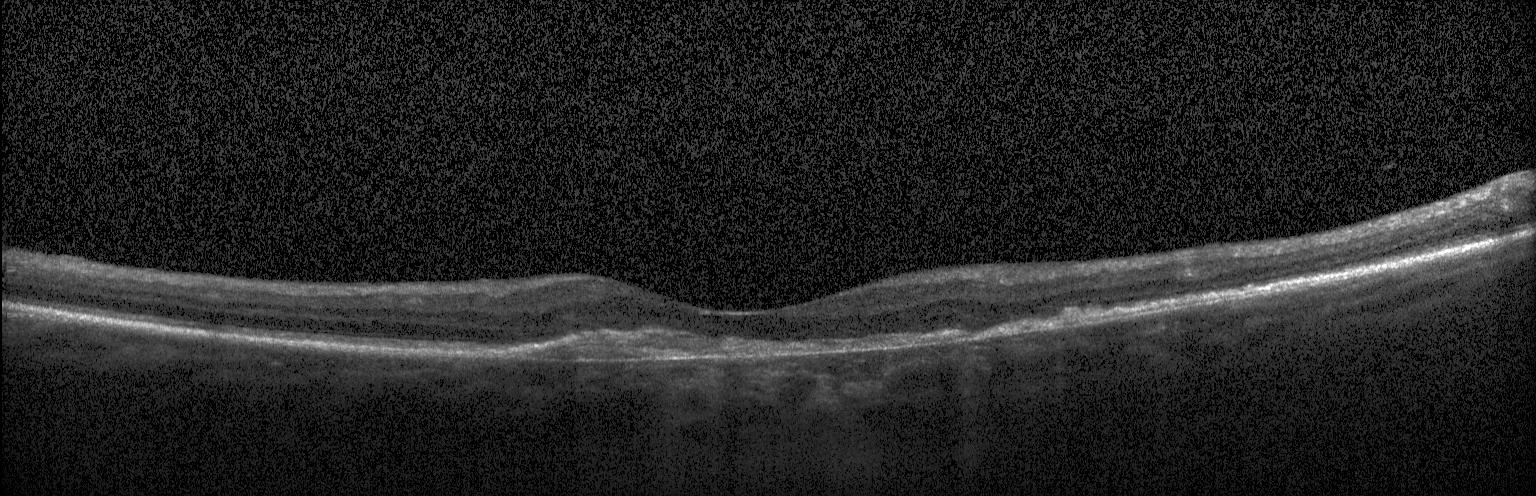
OCT B-scan.
This B-scan demonstrates choroidal neovascularization.